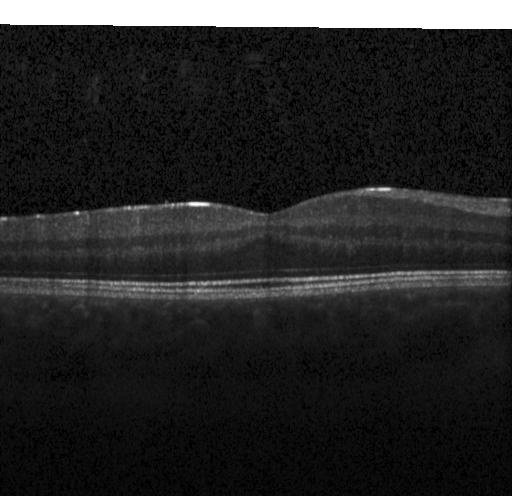

No evidence of choroidal neovascularization, diabetic macular edema, or drusen.